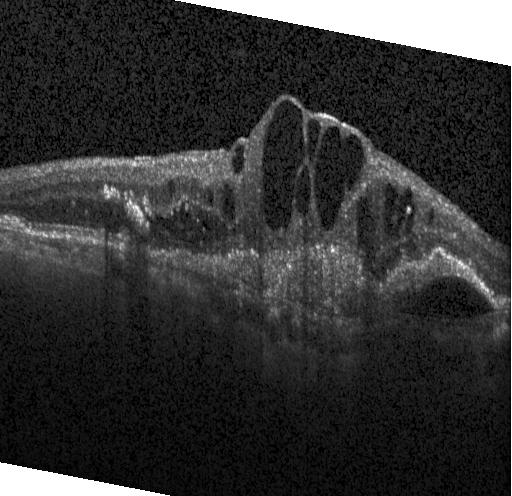
Finding: a choroidal neovascular membrane.